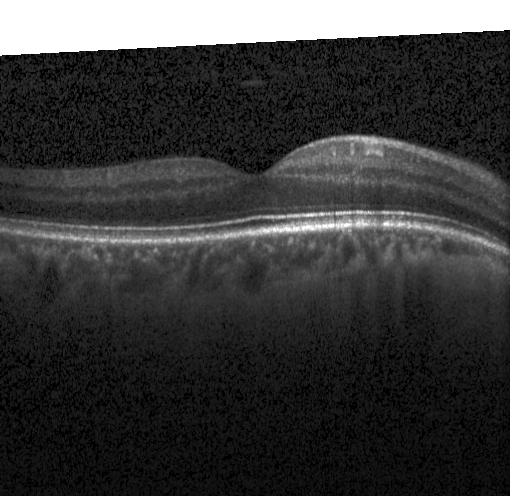
Optical coherence tomography scan — Finding: neither CNV, DME, nor drusen.